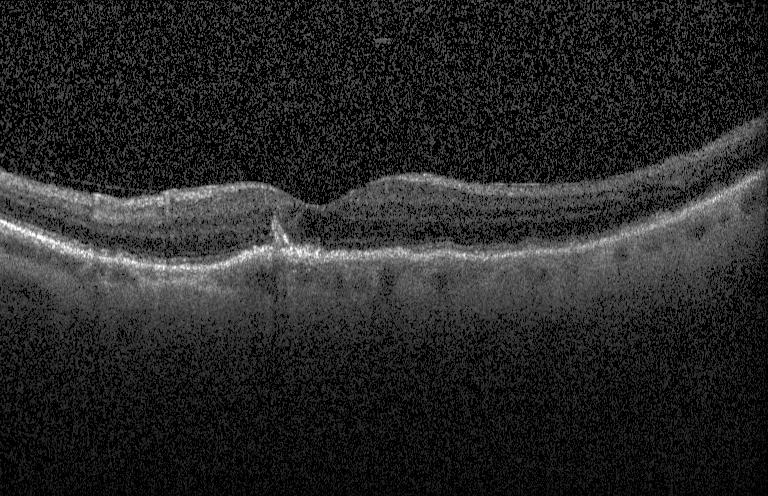
OCT line scan · macular scan
Finding: a choroidal neovascular membrane.